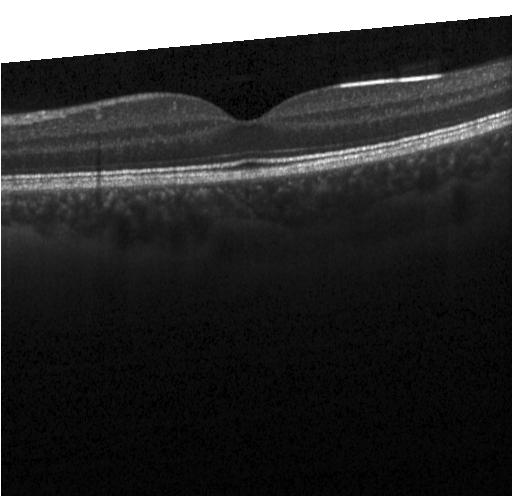
Acquired on a Heidelberg Spectralis, spectral-domain OCT, optical coherence tomography scan. No evidence of CNV, DME, or drusen.